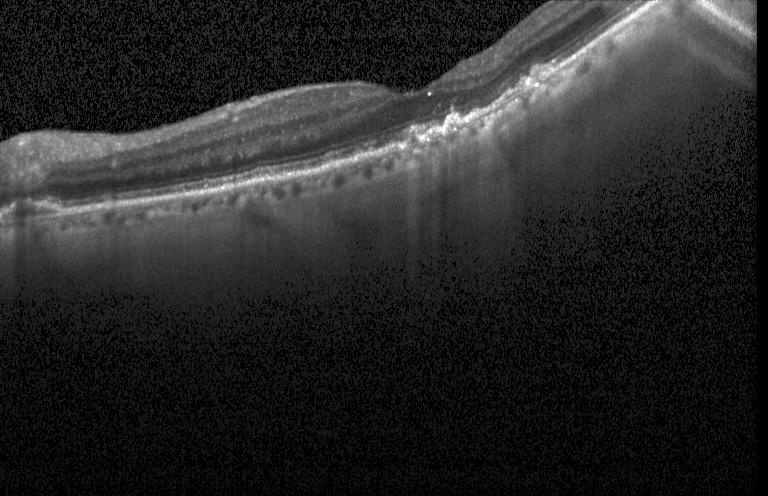

Dx: sub-RPE drusenoid deposits.